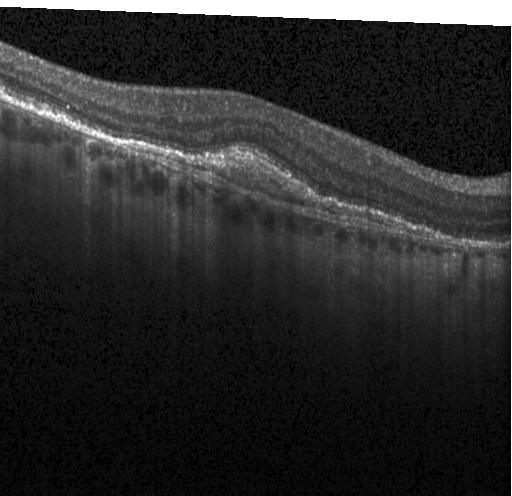 OCT scan showing a choroidal neovascular membrane.